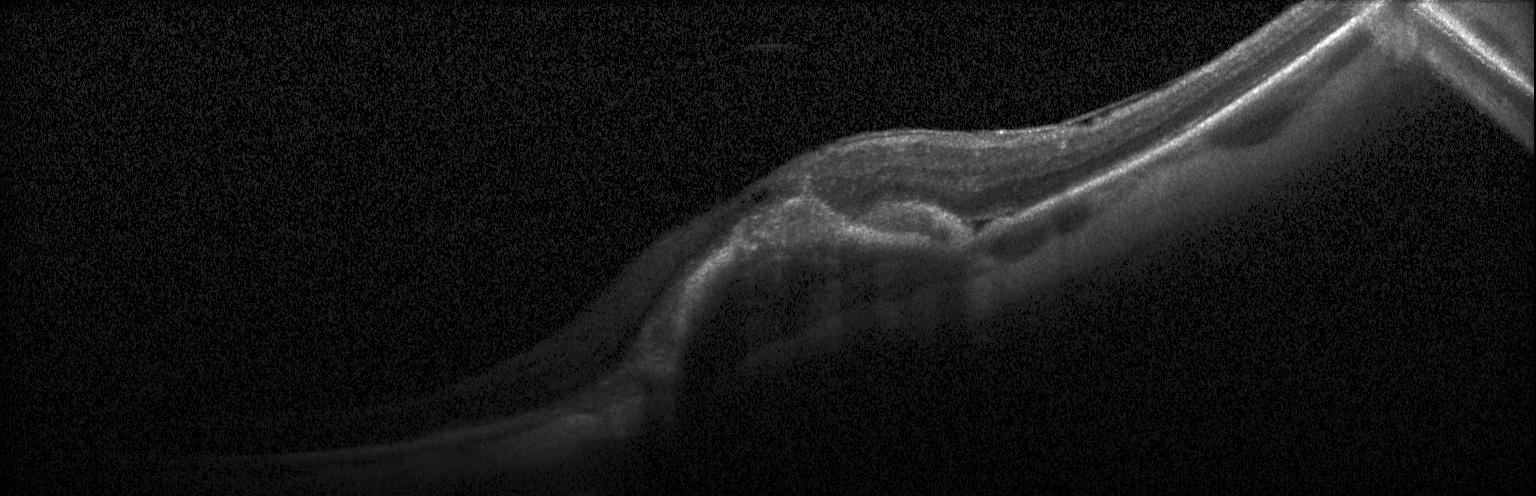 Fovea-centered. OCT B-scan. Spectral-domain OCT.
Impression: a choroidal neovascular membrane.